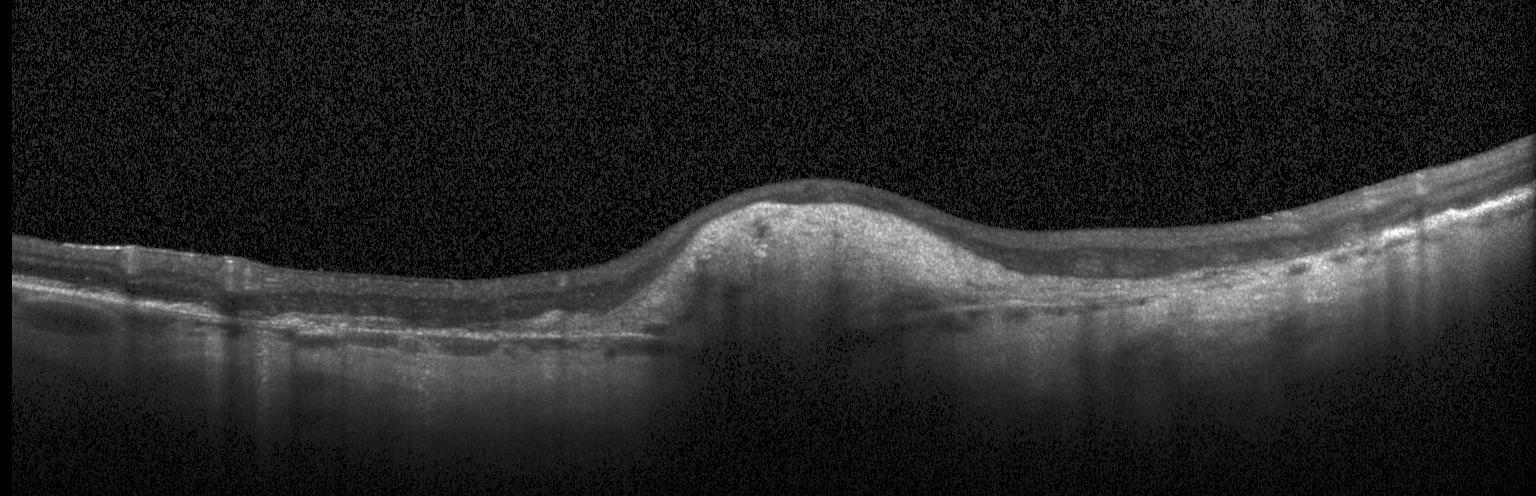 Optical coherence tomography B-scan
Dx: a choroidal neovascular membrane.